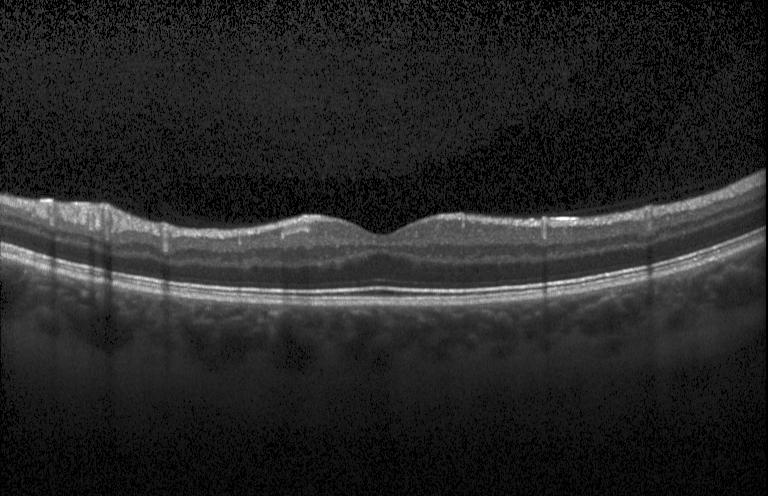 Heidelberg Spectralis; retinal OCT cross-section.
This B-scan demonstrates no CNV, no DME, and no drusen.